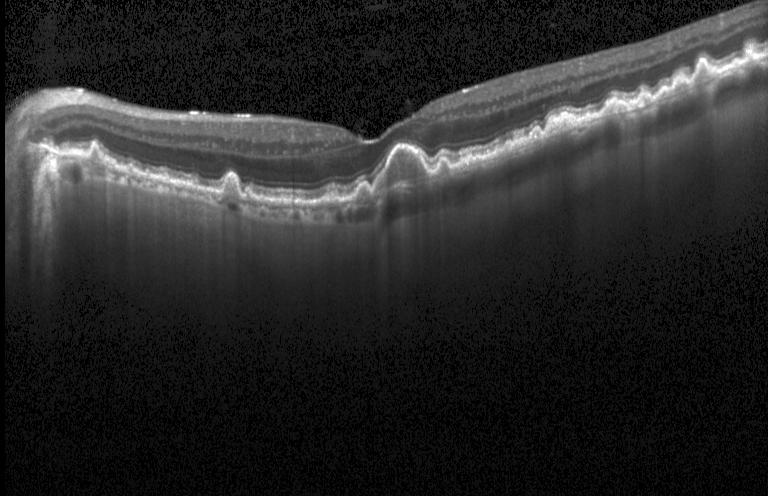

Retinal OCT cross-section. Assessment: multiple drusen.